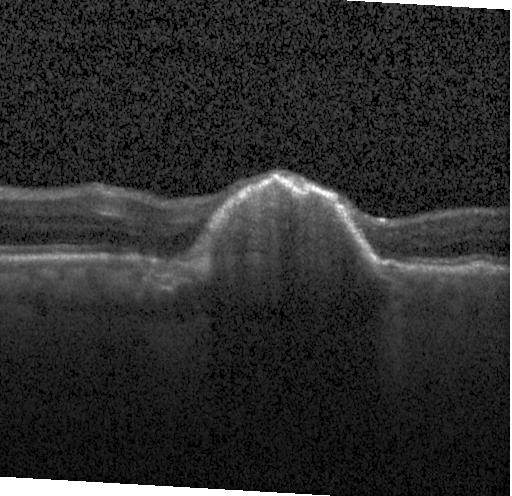

OCT line scan.
The scan shows CNV.